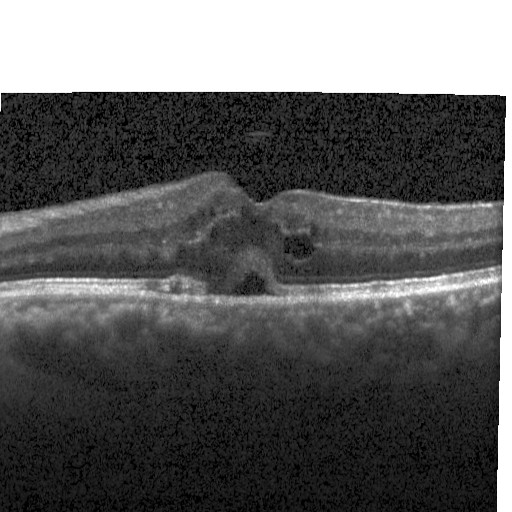
OCT finding: diabetic macular edema.